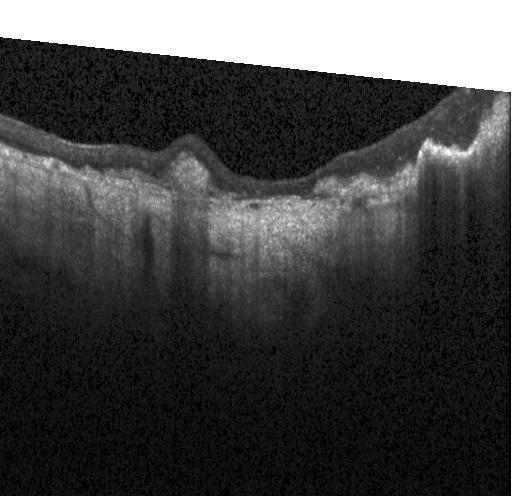 Dx: a choroidal neovascular membrane.